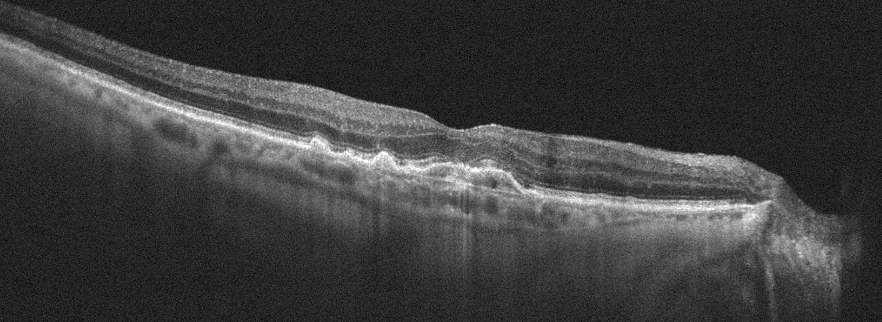

Macular scan. OCT line scan.
This B-scan demonstrates age-related macular degeneration.